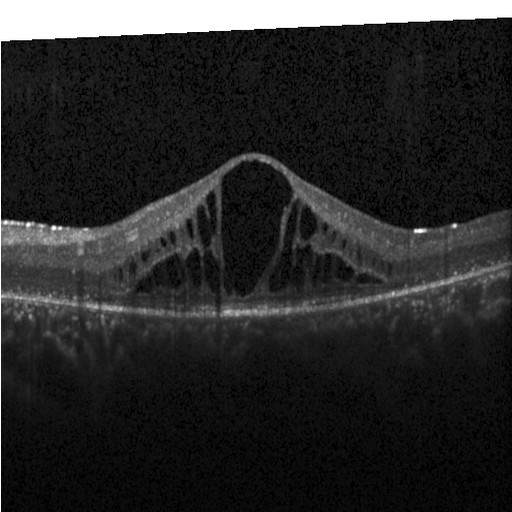 Macular OCT: diabetic macular edema (DME).